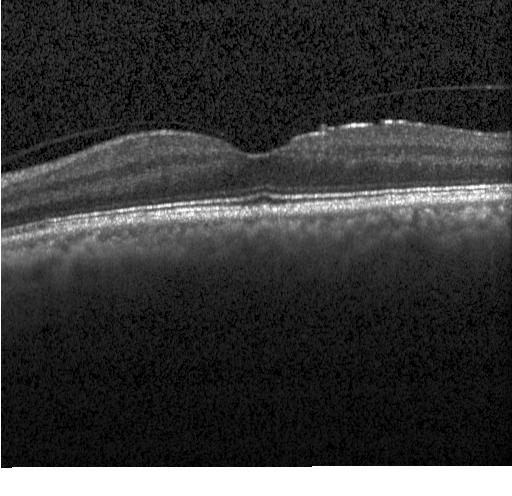

OCT scan showing no evidence of choroidal neovascularization, diabetic macular edema, or drusen.